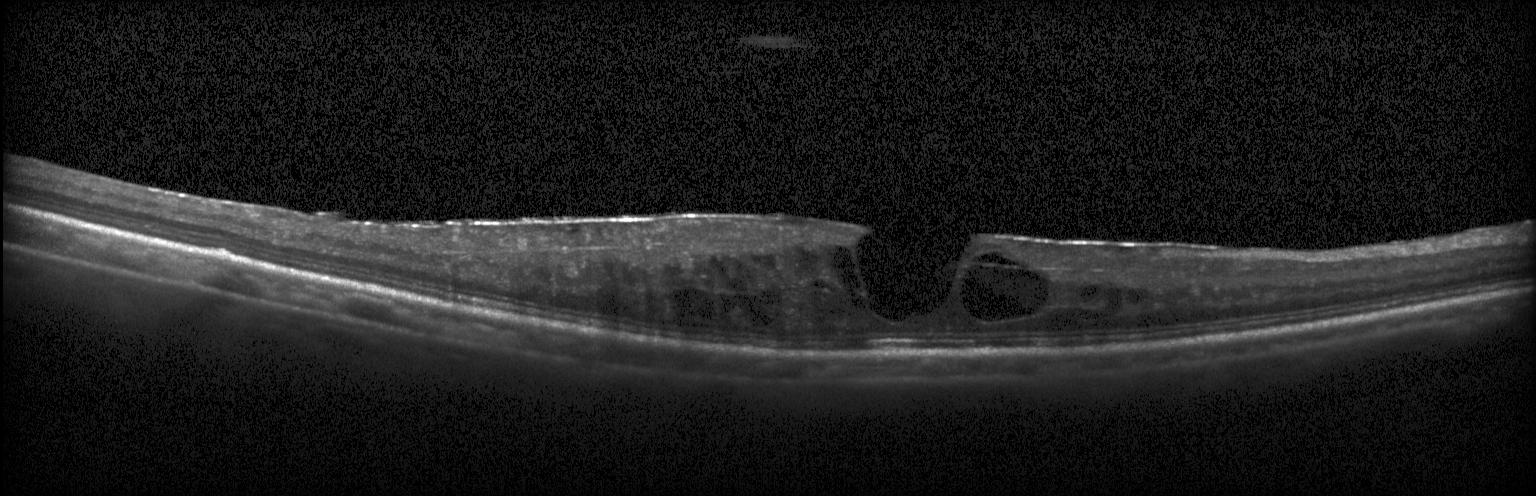

Heidelberg Spectralis OCT system, optical coherence tomography B-scan, through the macula.
OCT finding: DME.